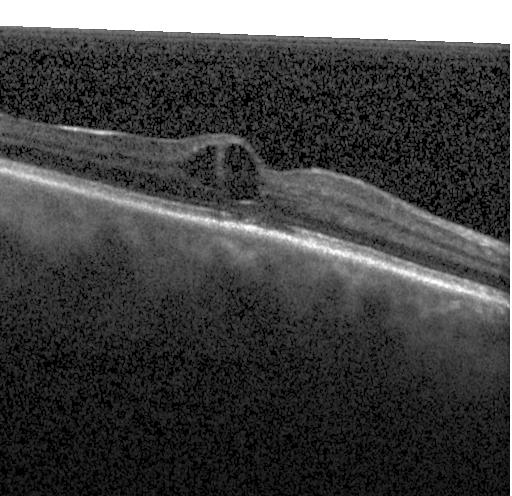 The scan shows diabetic macular edema.